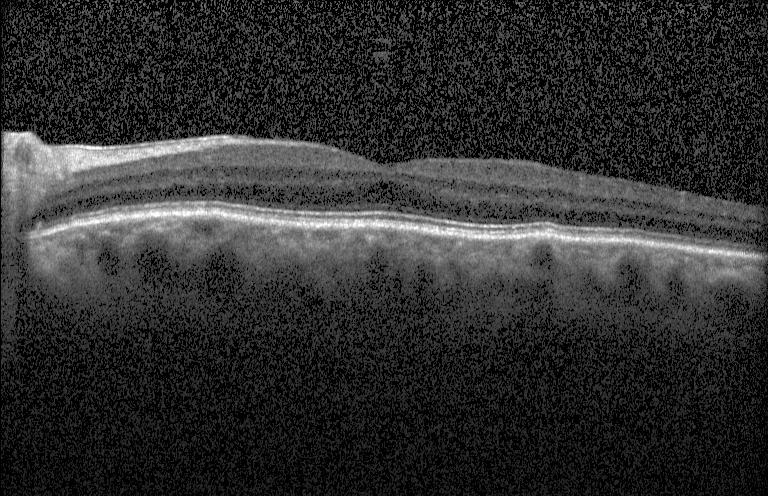 Fovea-centered, spectral-domain optical coherence tomography, Heidelberg Spectralis OCT system, OCT line scan
This B-scan demonstrates no evidence of CNV, DME, or drusen.